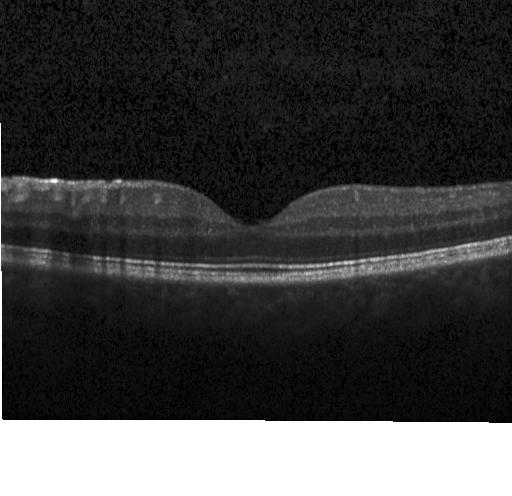 OCT scan showing neither CNV, DME, nor drusen.